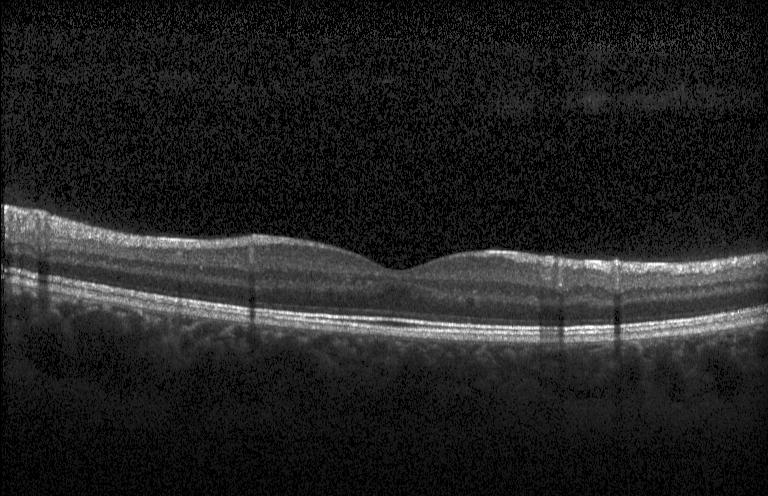

Retinal OCT B-scan; instrument: Heidelberg Spectralis; SD-OCT; centered on the fovea
The scan shows no CNV, no DME, and no drusen.